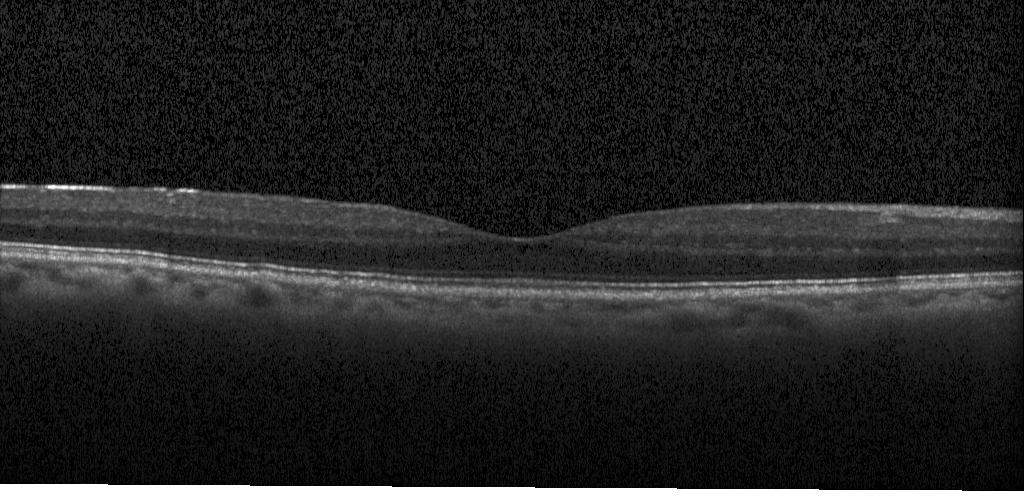
Macular OCT: no CNV, DME, or drusen.